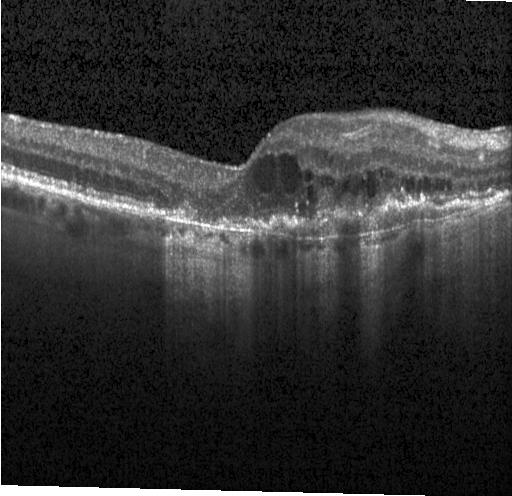

Impression: choroidal neovascularization (CNV).